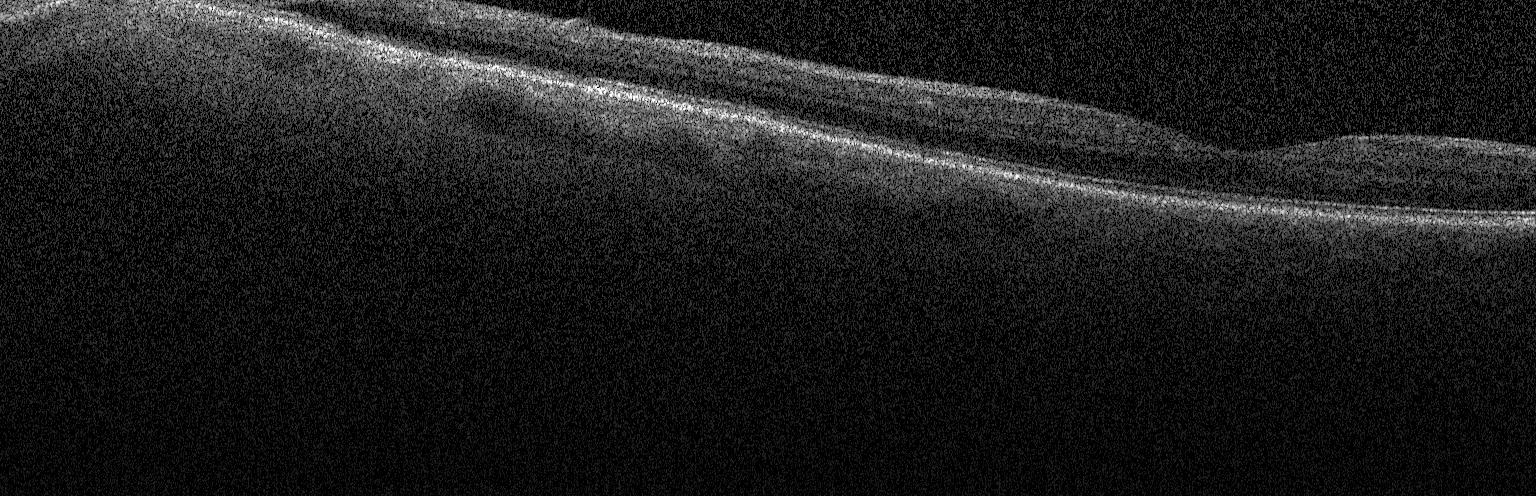

OCT B-scan · spectral-domain OCT · macular scan · acquired on a Heidelberg Spectralis. OCT finding: no choroidal neovascularization, no diabetic macular edema, and no drusen.